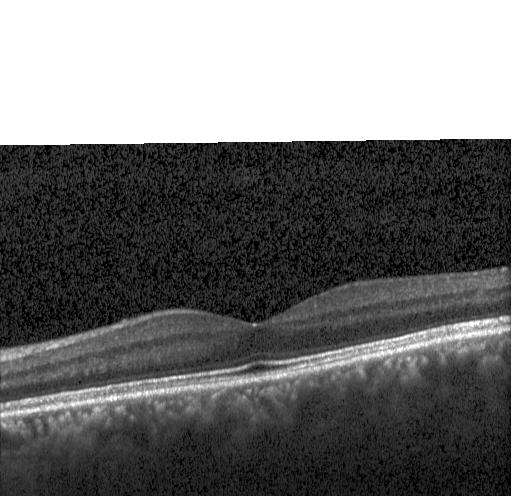
Macular OCT demonstrating no evidence of choroidal neovascularization, diabetic macular edema, or drusen.